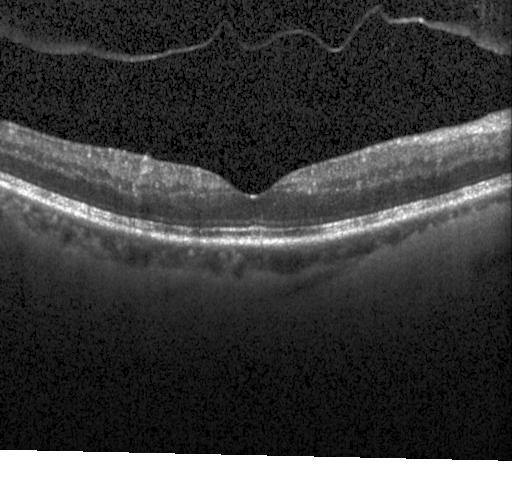

OCT B-scan, Heidelberg Spectralis OCT system — No choroidal neovascularization, no diabetic macular edema, and no drusen.